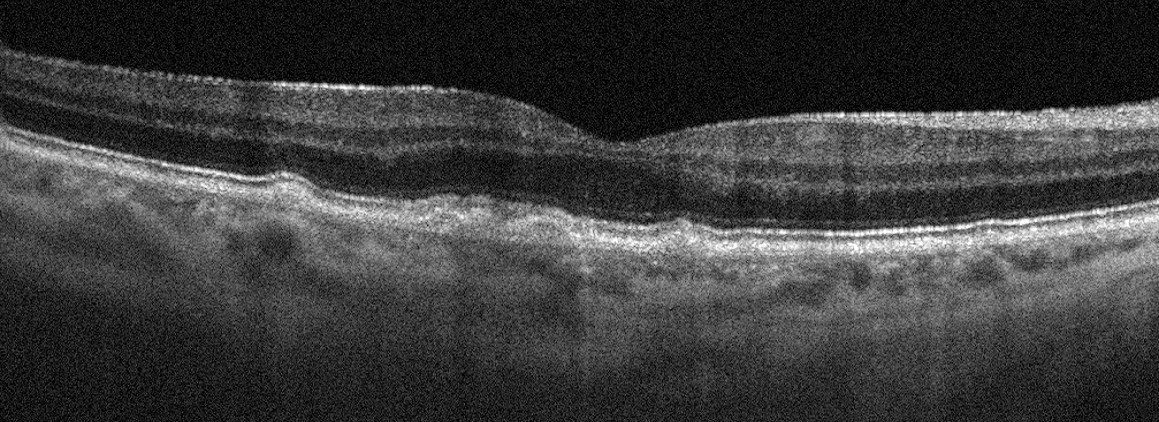 Acquired on an Optovue Avanti RTVue XR; optical coherence tomography B-scan; macular scan; OD
Finding: age-related macular degeneration.